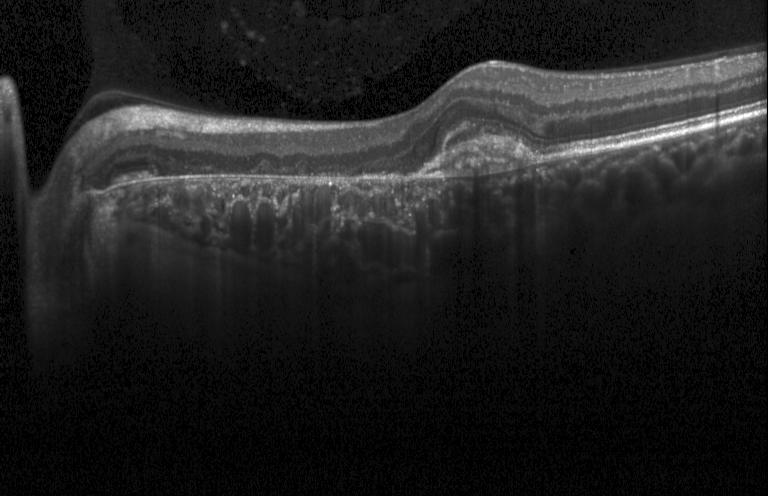 Retinal OCT cross-section; horizontal scan through the fovea; SD-OCT. Impression: choroidal neovascularization.